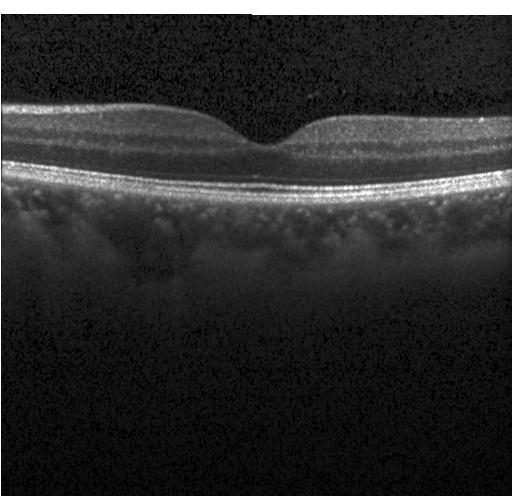
Retinal OCT cross-section. The scan shows no evidence of CNV, DME, or drusen.